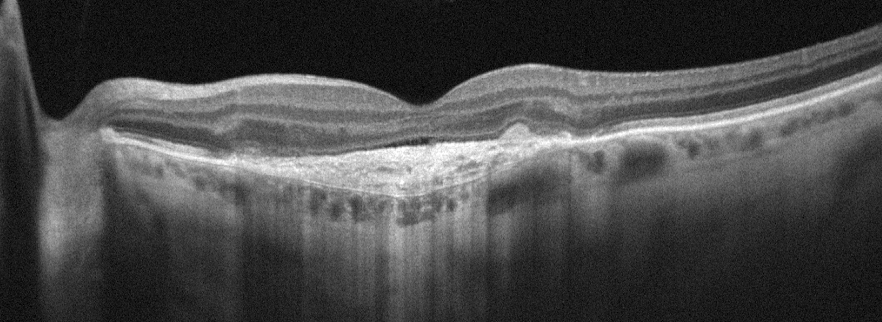

Instrument: Optovue Avanti RTVue XR. Retinal OCT cross-section. Through the macula. Oculus sinister
OCT finding: age-related macular degeneration (AMD).